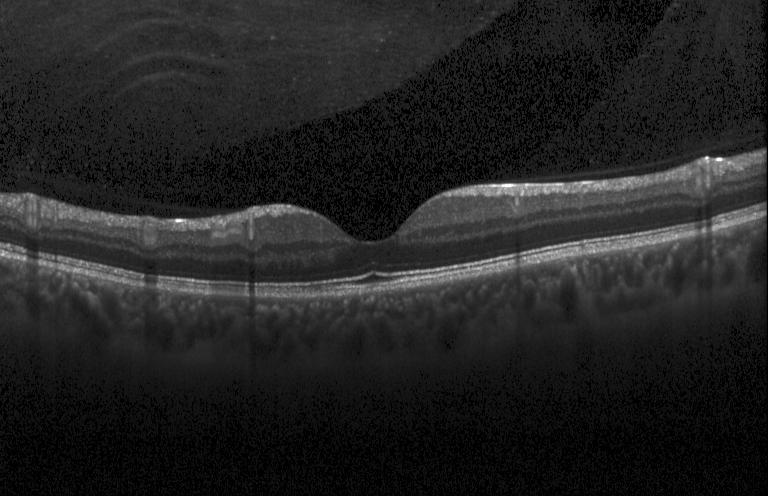 Dx: no choroidal neovascularization, no diabetic macular edema, and no drusen.